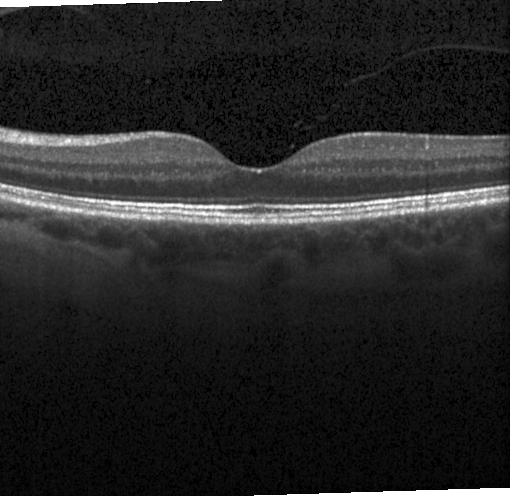
Optical coherence tomography B-scan — Dx: no evidence of choroidal neovascularization, diabetic macular edema, or drusen.